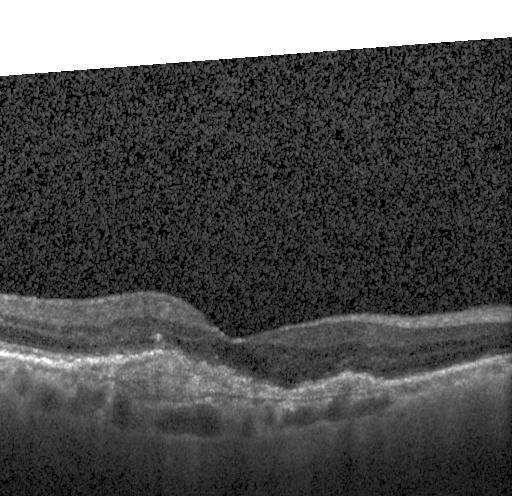

Retinal OCT cross-section showing a choroidal neovascular membrane.